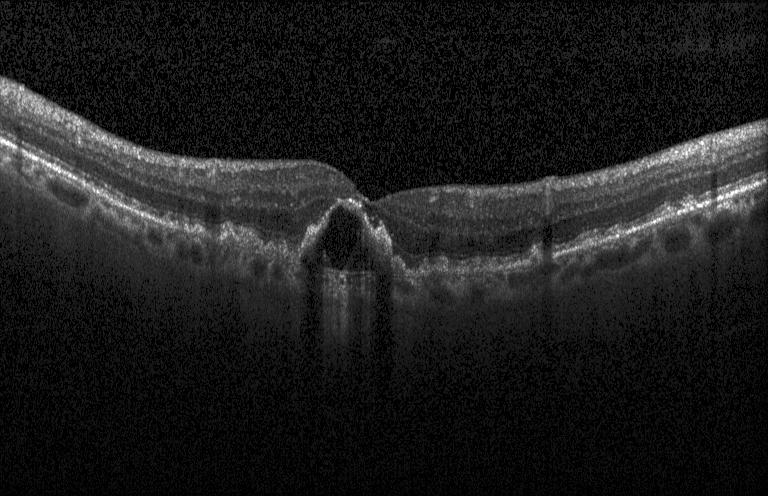
OCT B-scan · SD-OCT
Diagnosis: a choroidal neovascular membrane.